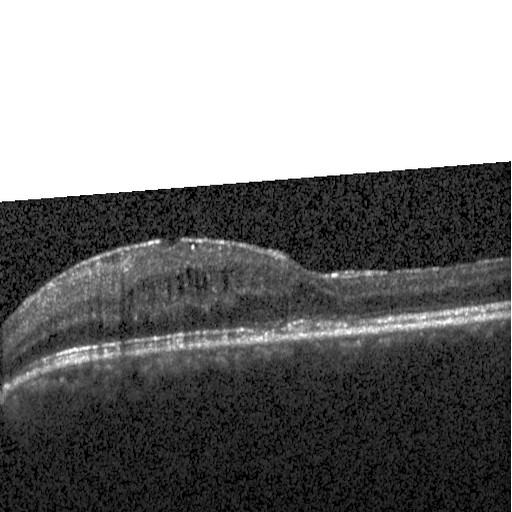

Macular OCT: DME.